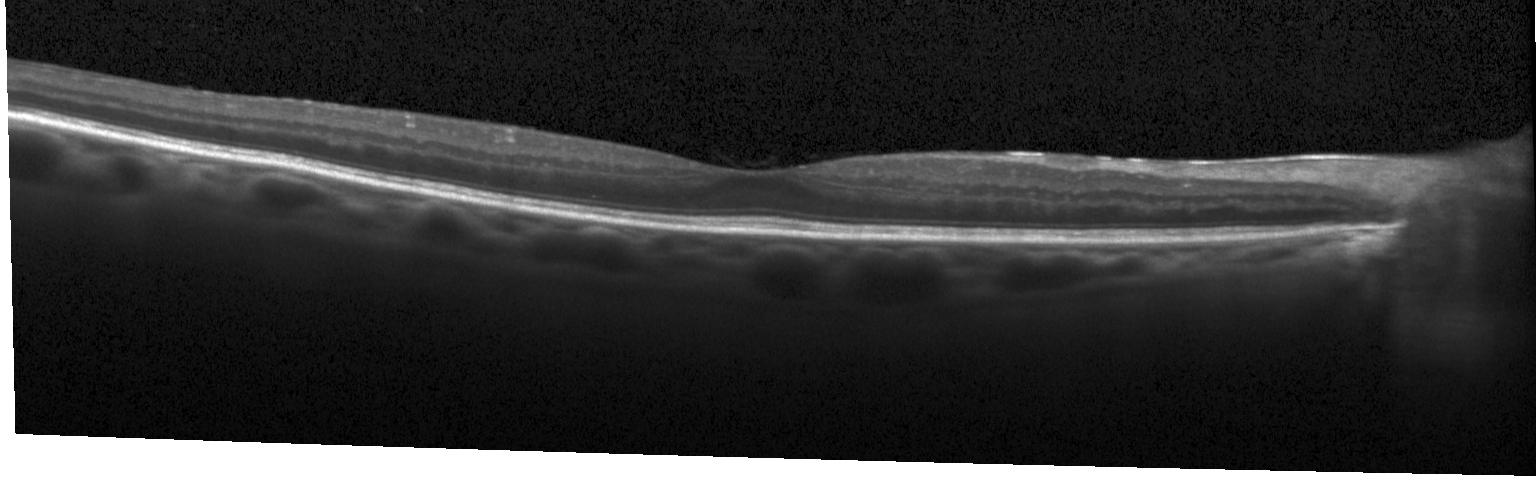

SD-OCT · Heidelberg Spectralis OCT system · optical coherence tomography B-scan
This B-scan demonstrates neither choroidal neovascularization, diabetic macular edema, nor drusen.